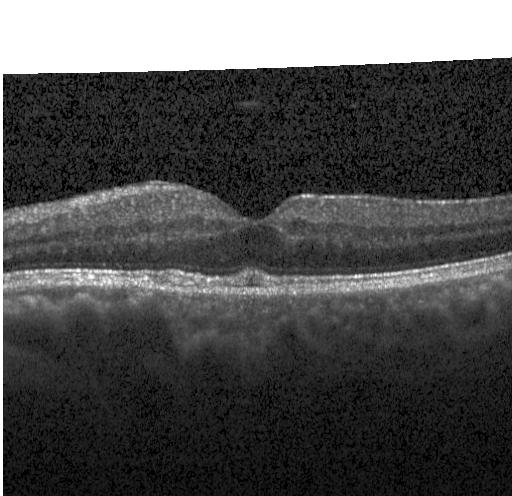 SD-OCT · OCT line scan — Diagnosis: neither choroidal neovascularization, diabetic macular edema, nor drusen.